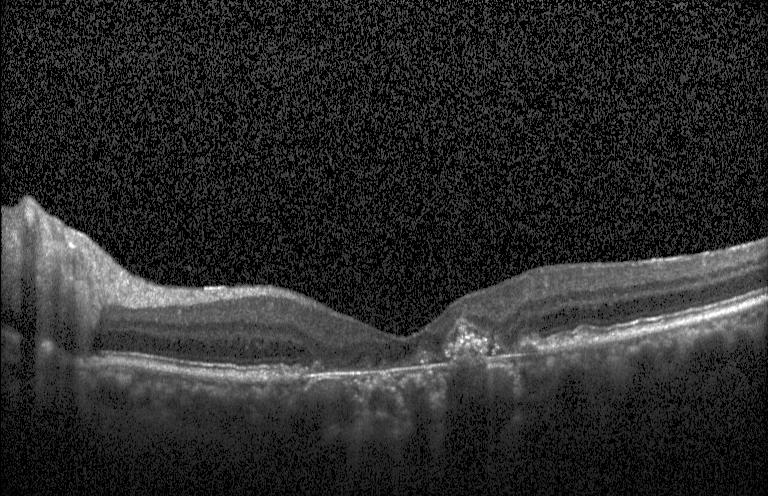
Finding: a choroidal neovascular membrane.